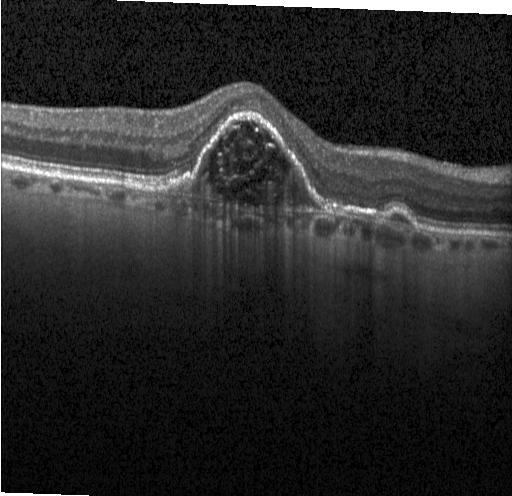

Macular OCT demonstrating CNV.